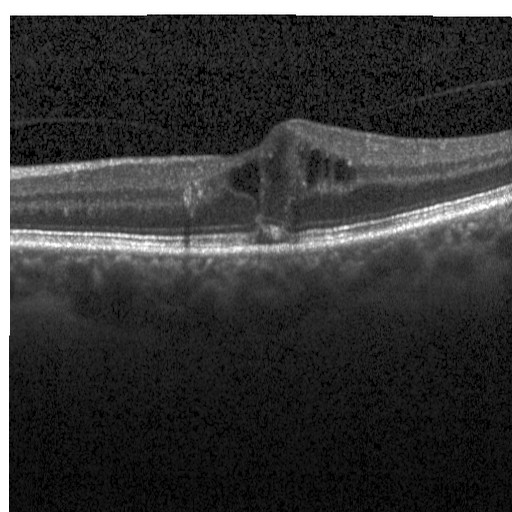 OCT line scan; instrument: Heidelberg Spectralis. Assessment: DME.